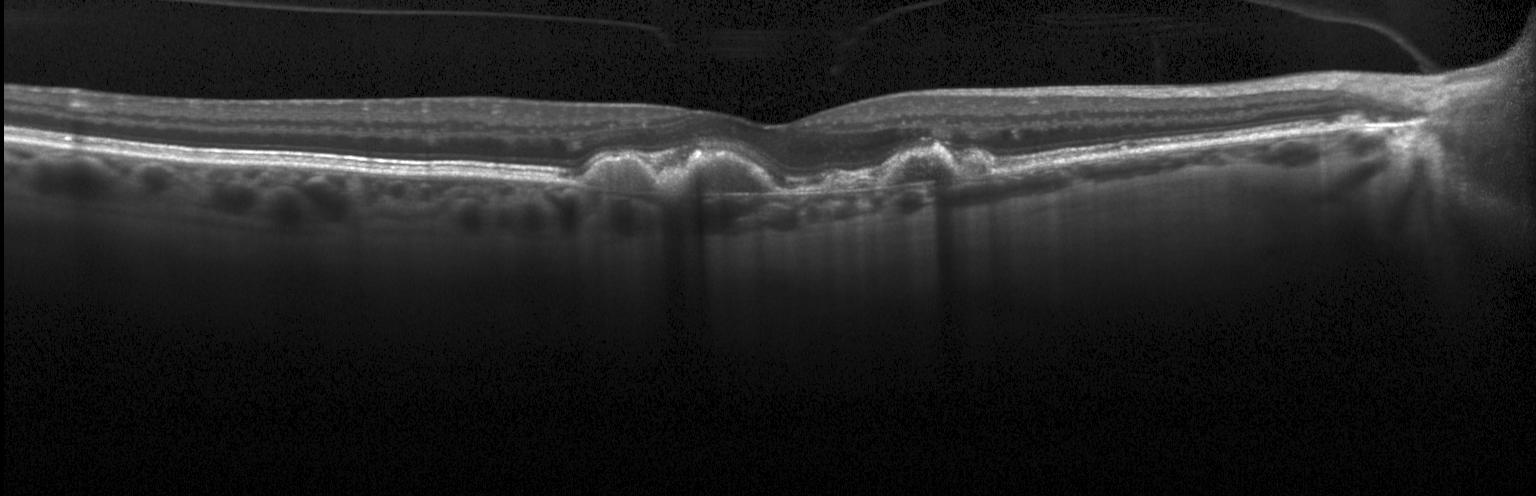

Retinal OCT cross-section — Macular OCT: choroidal neovascularization (CNV).